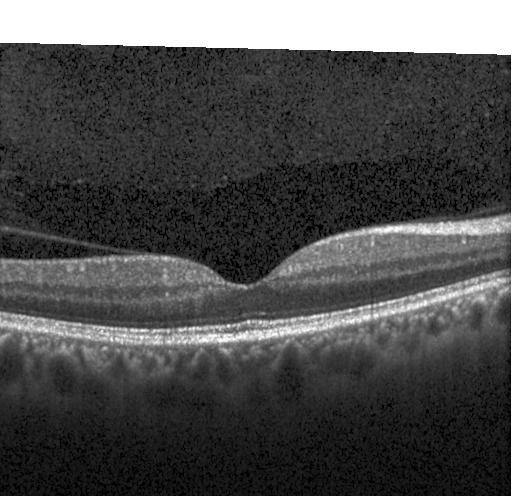 Finding: no evidence of CNV, DME, or drusen.